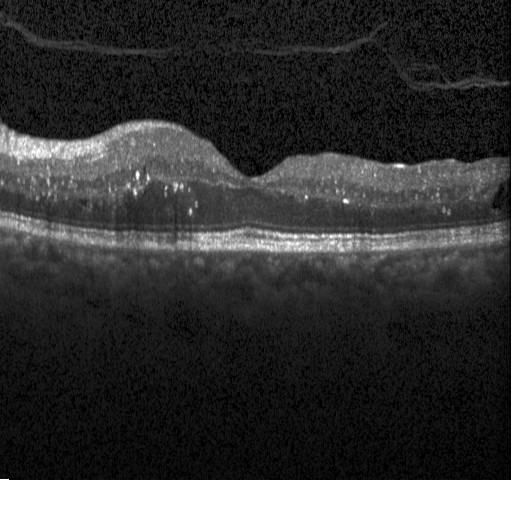 Heidelberg Spectralis, OCT line scan
Finding: diabetic macular edema (DME).